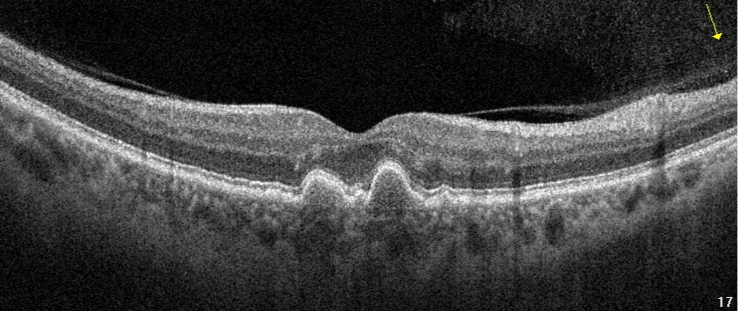
Acquired on an Optovue Avanti RTVue XR, OCT line scan, through the macula. Finding: age-related macular degeneration (AMD).